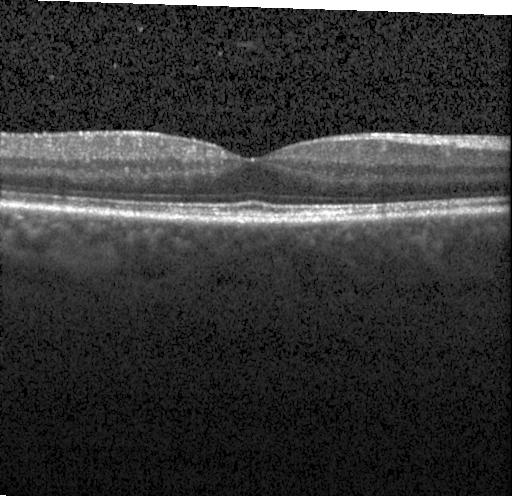 Retinal OCT cross-section — Dx: no choroidal neovascularization, no diabetic macular edema, and no drusen.